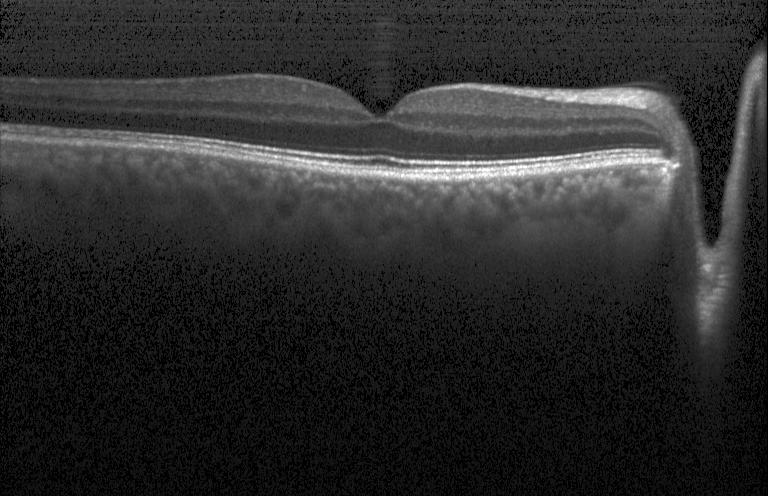

Optical coherence tomography B-scan
No CNV, no DME, and no drusen.